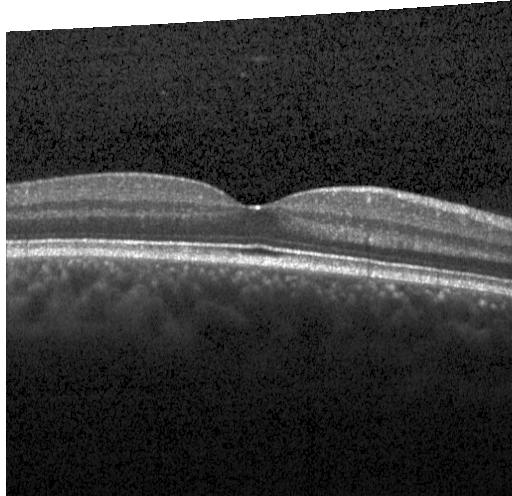
Optical coherence tomography B-scan — This B-scan demonstrates no CNV, no DME, and no drusen.